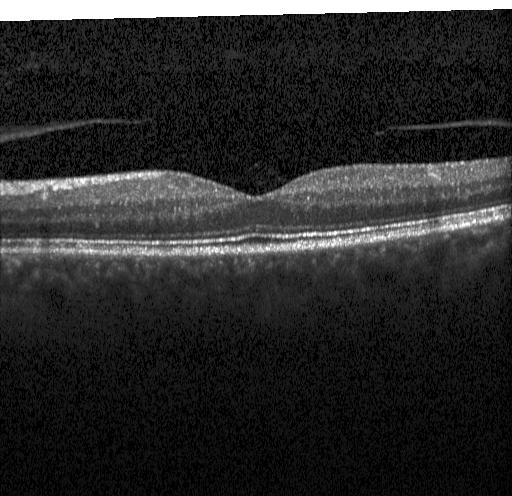
Horizontal scan through the fovea; spectral-domain optical coherence tomography; retinal OCT cross-section; acquired on a Heidelberg Spectralis. Finding: neither choroidal neovascularization, diabetic macular edema, nor drusen.